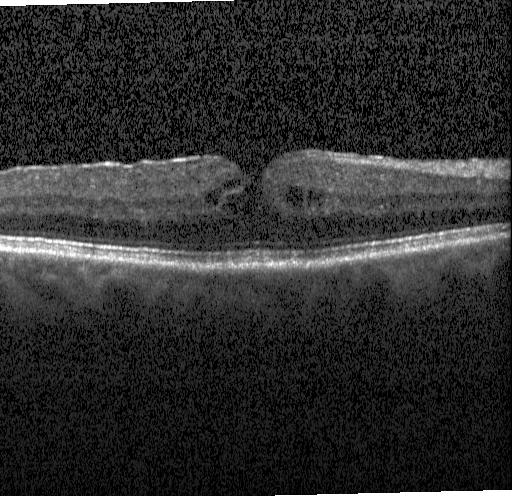
Acquired on a Heidelberg Spectralis. Spectral-domain optical coherence tomography. Optical coherence tomography scan. Through the macula. Finding: diabetic macular edema.